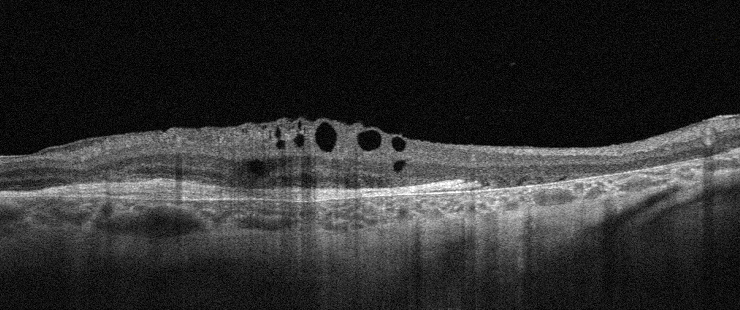
Optical coherence tomography B-scan — Age-related macular degeneration (AMD).